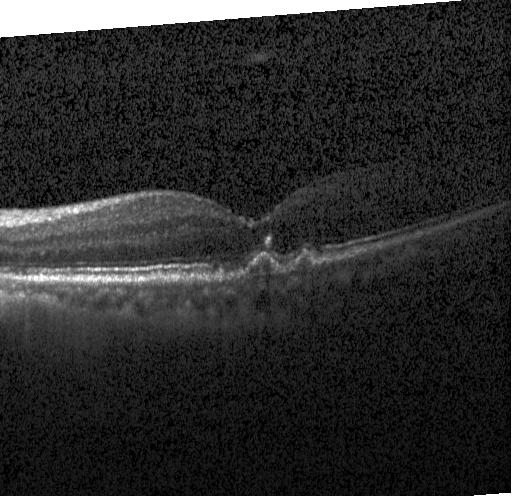 Macular scan; retinal OCT cross-section; acquired on a Heidelberg Spectralis; spectral-domain optical coherence tomography.
Sub-RPE drusenoid deposits.